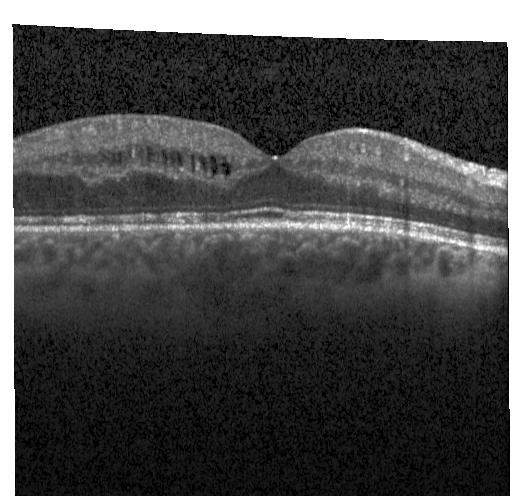
Assessment: DME.